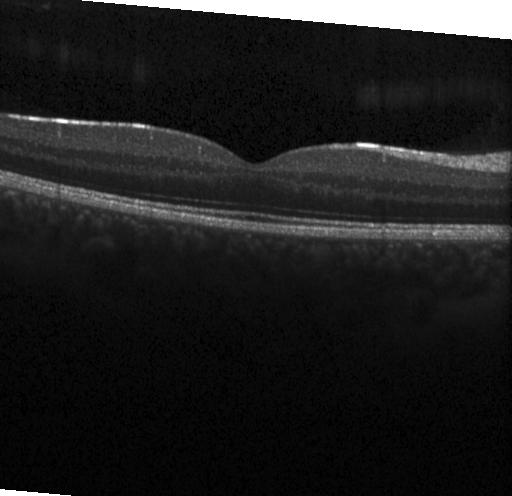

Impression: no evidence of choroidal neovascularization, diabetic macular edema, or drusen.